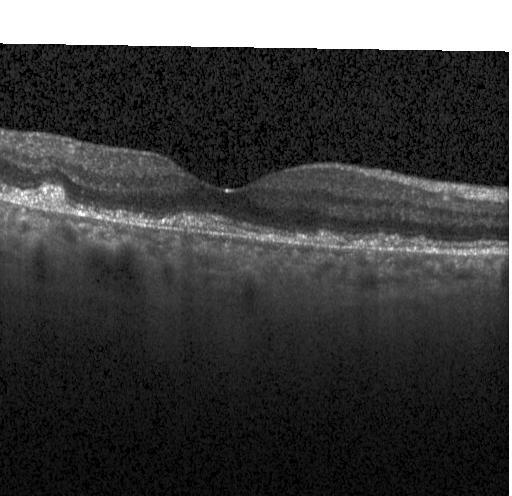 This B-scan demonstrates CNV.